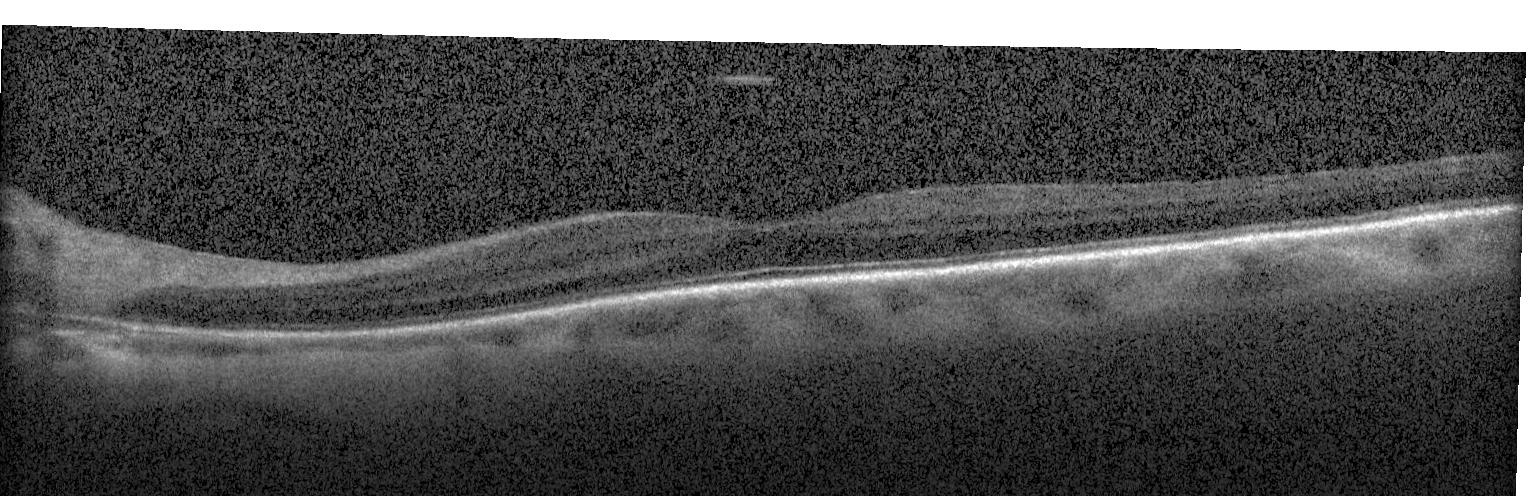

Retinal OCT B-scan, spectral-domain OCT, acquired on a Heidelberg Spectralis.
Diagnosis: no choroidal neovascularization, diabetic macular edema, or drusen.